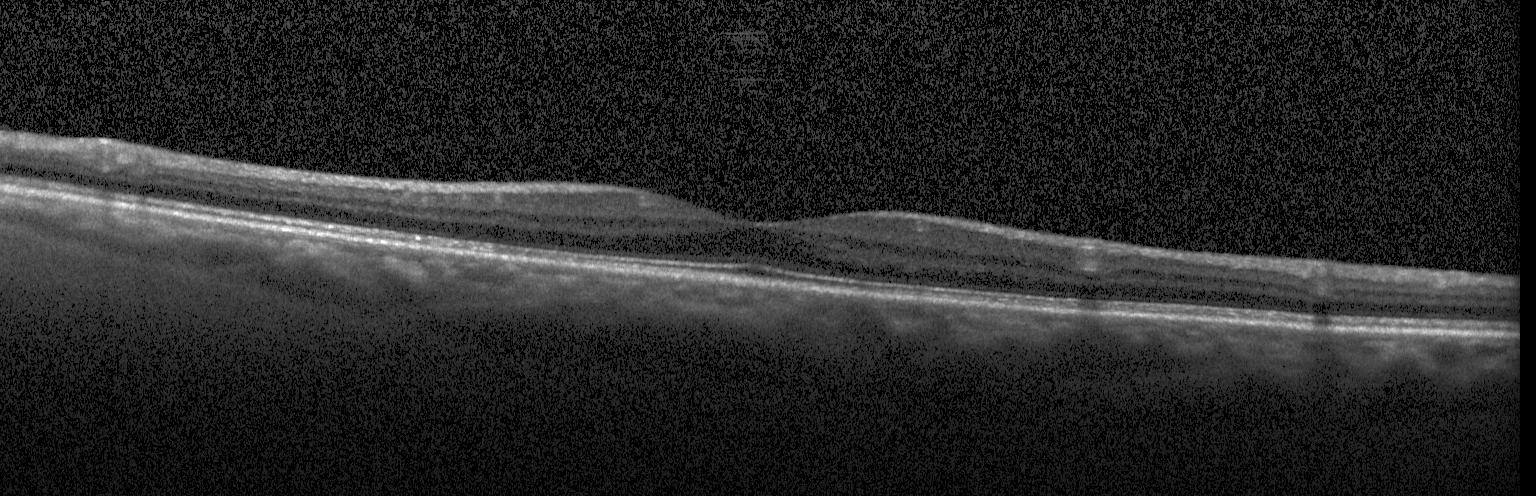
Optical coherence tomography scan, centered on the fovea, instrument: Heidelberg Spectralis
Dx: no evidence of CNV, DME, or drusen.